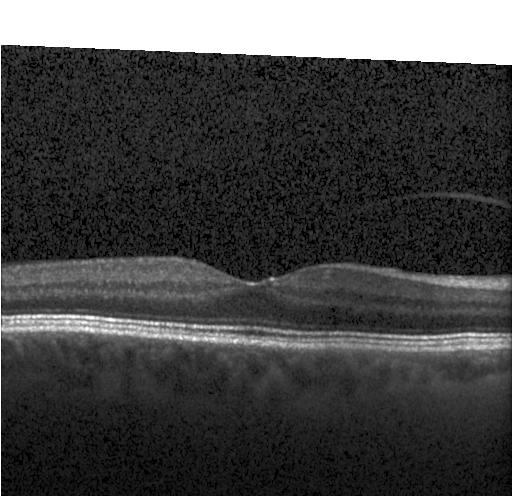
Finding: neither CNV, DME, nor drusen.